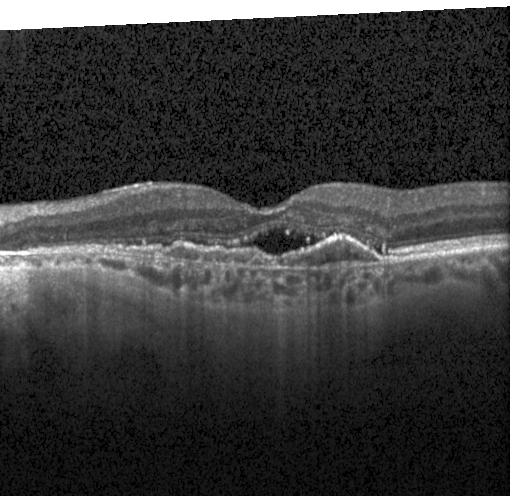
OCT line scan. Heidelberg Spectralis OCT system. SD-OCT. Centered on the fovea
Impression: a choroidal neovascular membrane.